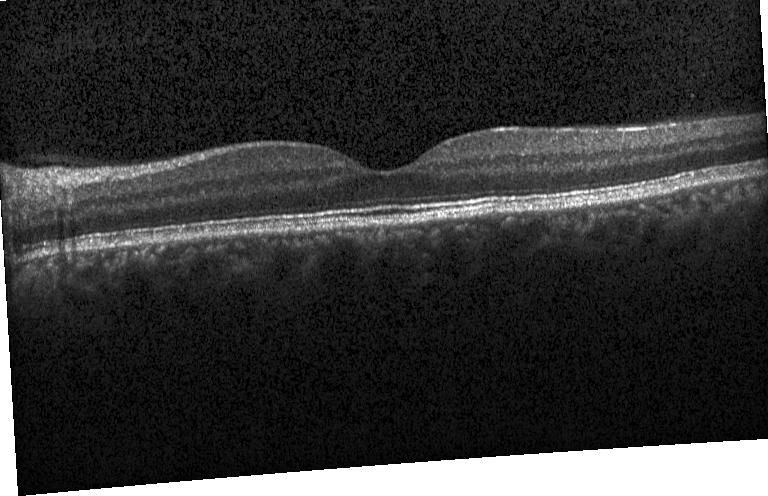 Retinal OCT B-scan; fovea-centered
Diagnosis: no evidence of CNV, DME, or drusen.